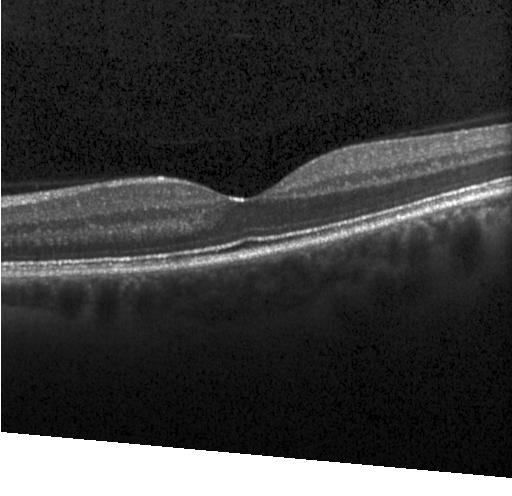
OCT finding: neither CNV, DME, nor drusen.